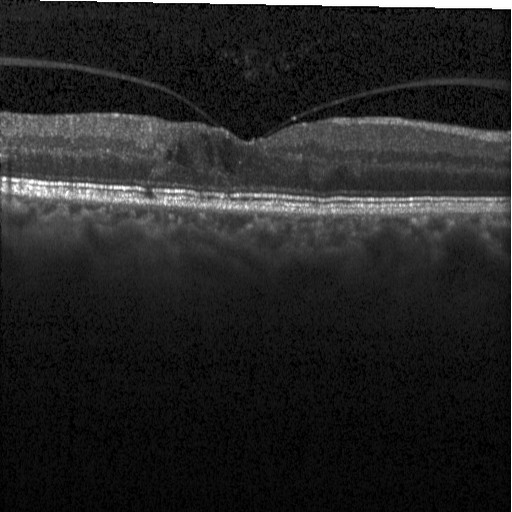 OCT B-scan · Heidelberg Spectralis
Diagnosis: diabetic macular edema.